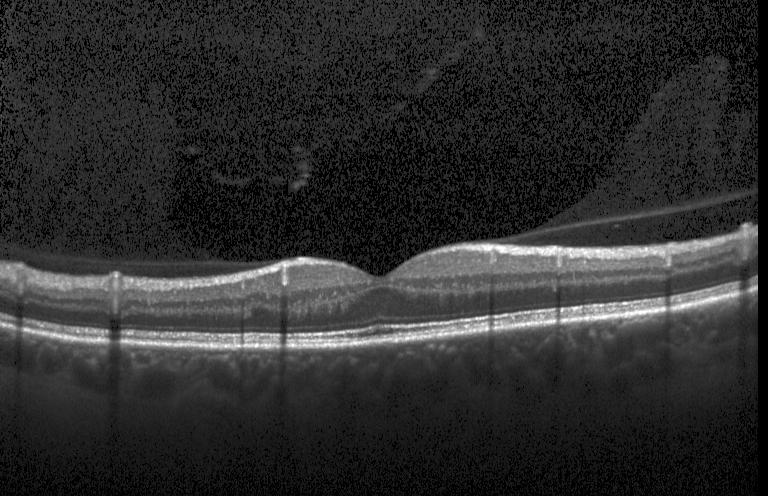
Optical coherence tomography B-scan.
Diagnosis: no CNV, DME, or drusen.